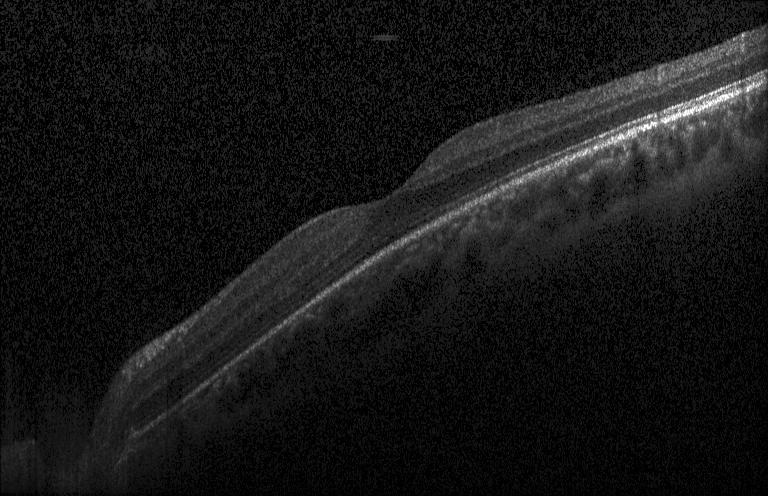
Retinal OCT cross-section. Impression: no choroidal neovascularization, diabetic macular edema, or drusen.